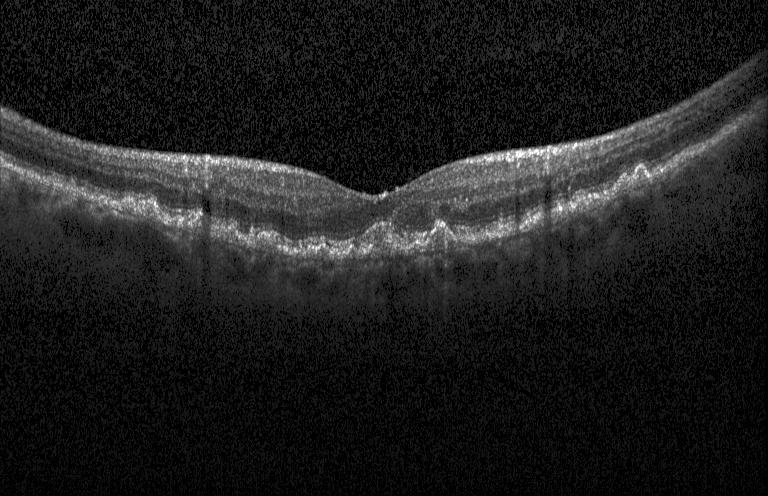 Retinal OCT cross-section — Assessment: sub-RPE drusenoid deposits.